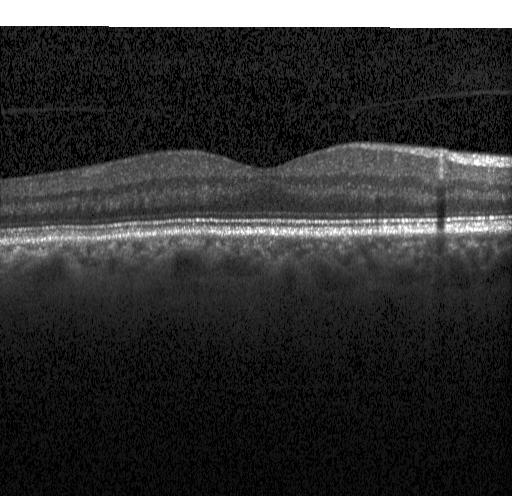
Impression: neither CNV, DME, nor drusen.